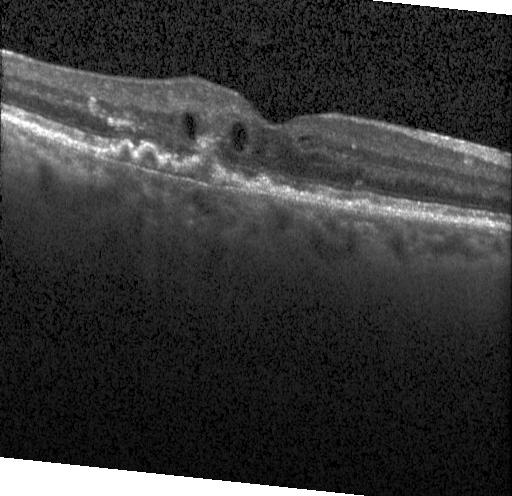

Heidelberg Spectralis OCT system; optical coherence tomography scan
Finding: a choroidal neovascular membrane.